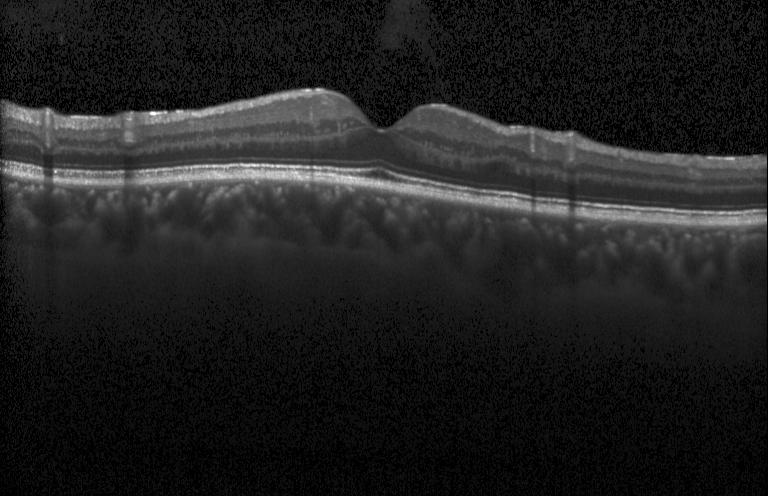
Optical coherence tomography scan; spectral-domain optical coherence tomography. Dx: no evidence of CNV, DME, or drusen.